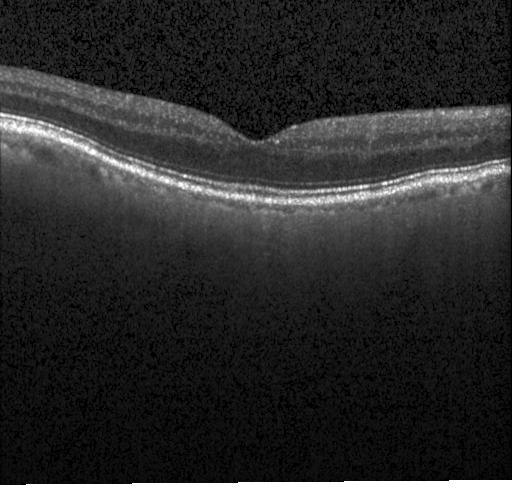

OCT finding: no choroidal neovascularization, diabetic macular edema, or drusen.